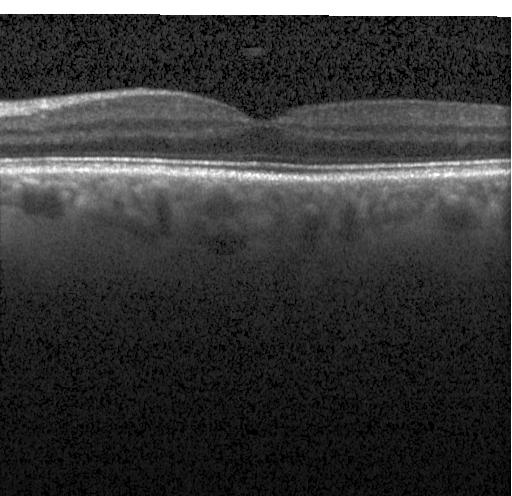
Dx: no choroidal neovascularization, no diabetic macular edema, and no drusen.